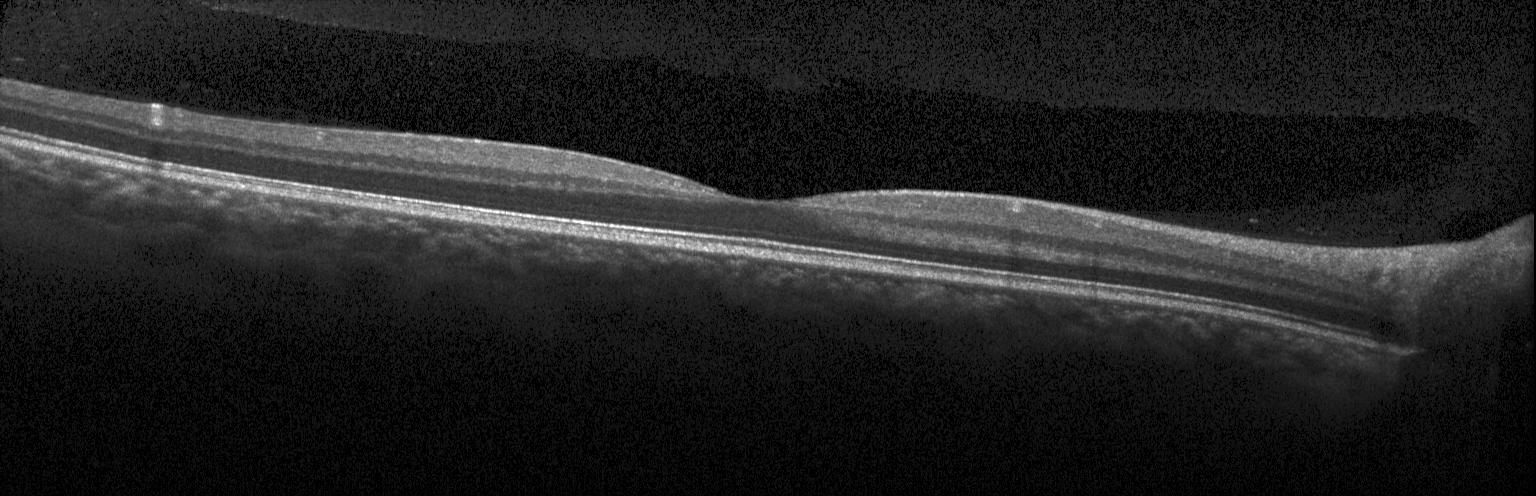
Instrument: Heidelberg Spectralis; optical coherence tomography B-scan. Neither choroidal neovascularization, diabetic macular edema, nor drusen.